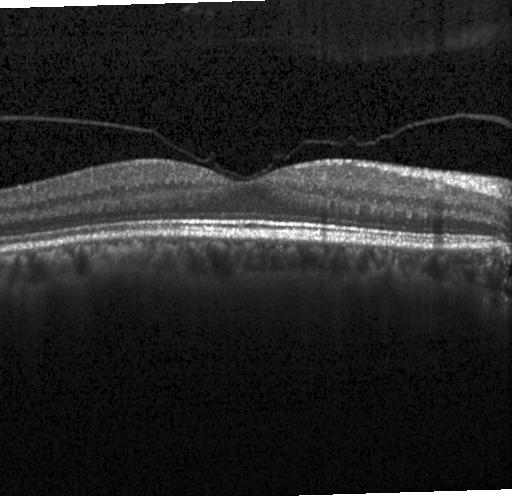 Macular scan, retinal OCT cross-section, Heidelberg Spectralis OCT system, SD-OCT. Impression: no choroidal neovascularization, diabetic macular edema, or drusen.